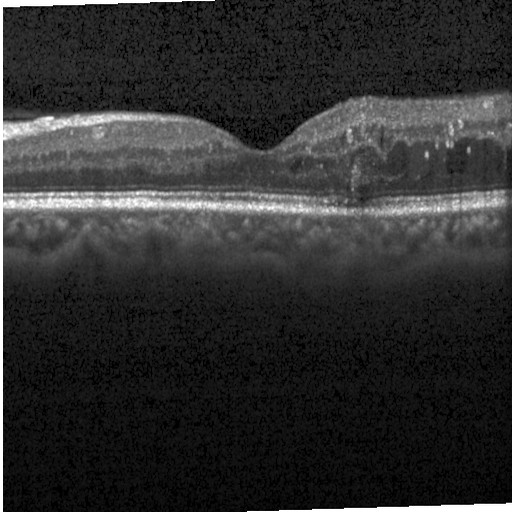
OCT B-scan showing DME.